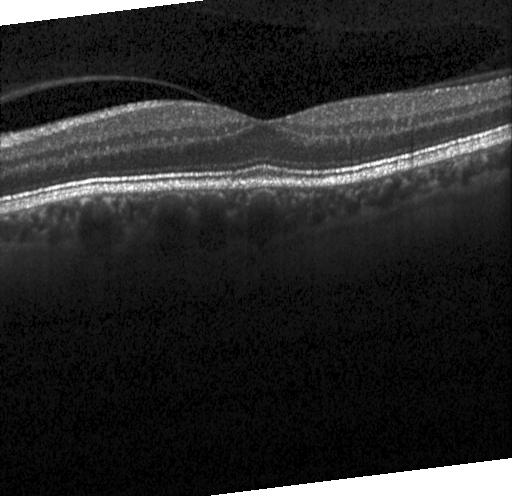 OCT line scan
Impression: no choroidal neovascularization, no diabetic macular edema, and no drusen.